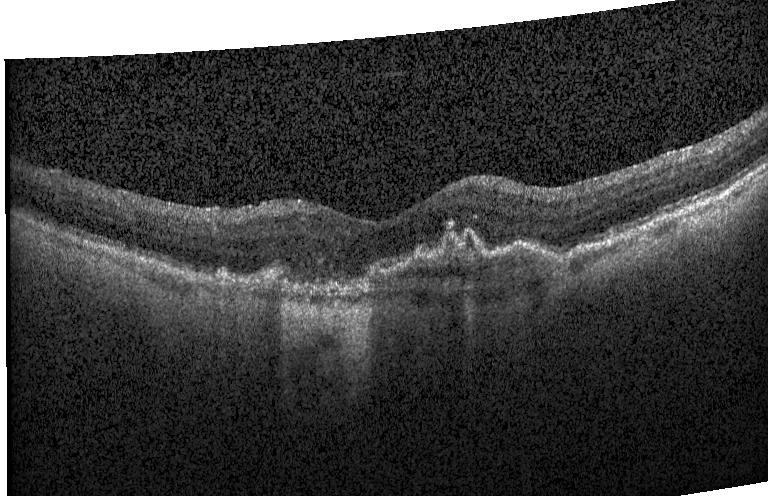

Optical coherence tomography B-scan
Diagnosis: choroidal neovascularization (CNV).